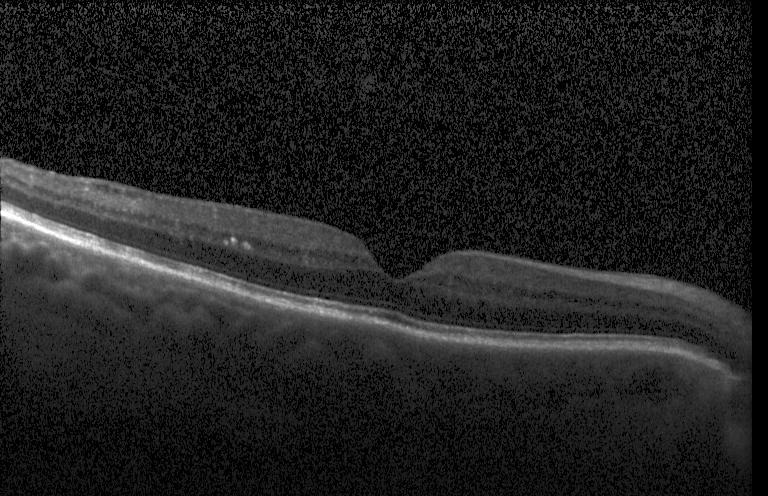 Macular OCT: no choroidal neovascularization, diabetic macular edema, or drusen.